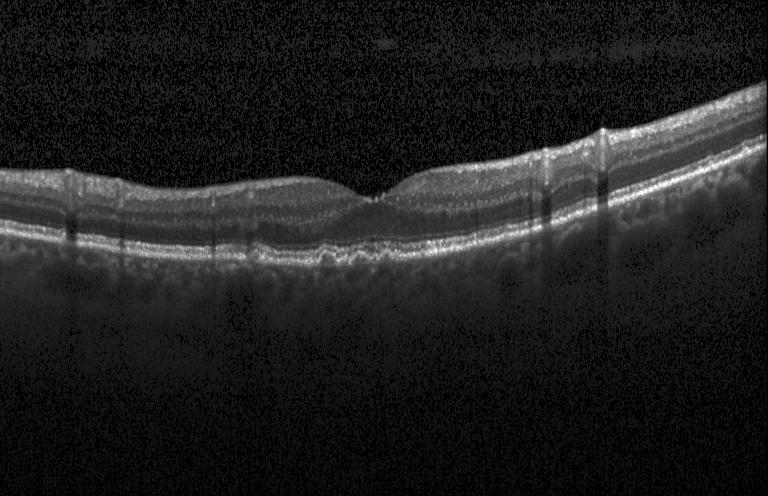
Retinal OCT cross-section, through the macula. OCT finding: drusen.